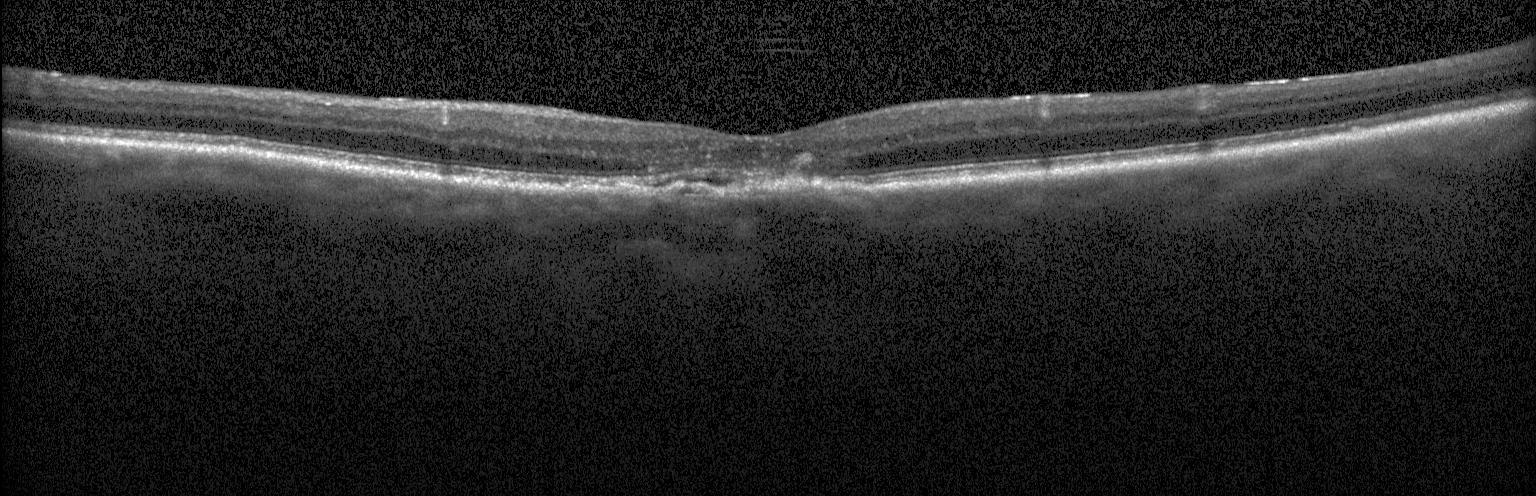

Heidelberg Spectralis; retinal OCT cross-section; through the macula. This B-scan demonstrates a choroidal neovascular membrane.